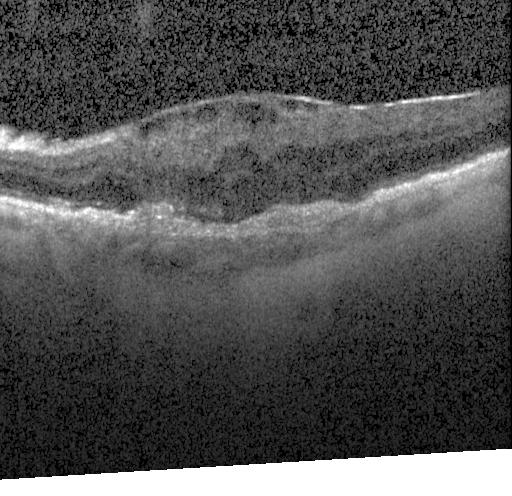
This B-scan demonstrates a choroidal neovascular membrane.